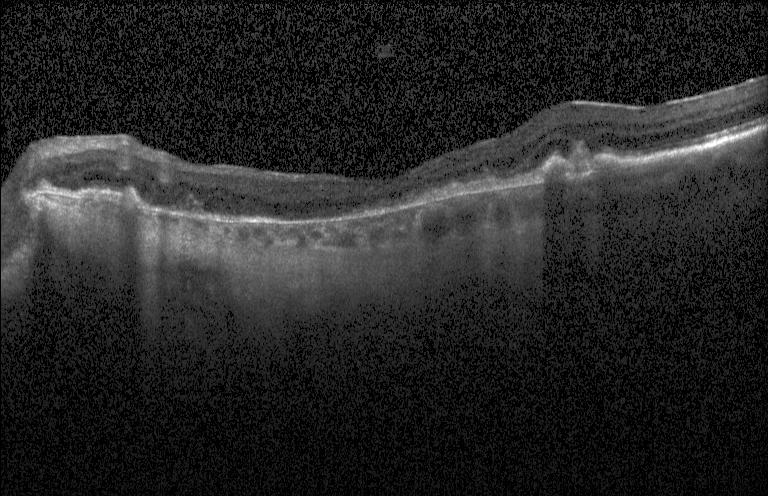
OCT B-scan showing a choroidal neovascular membrane.